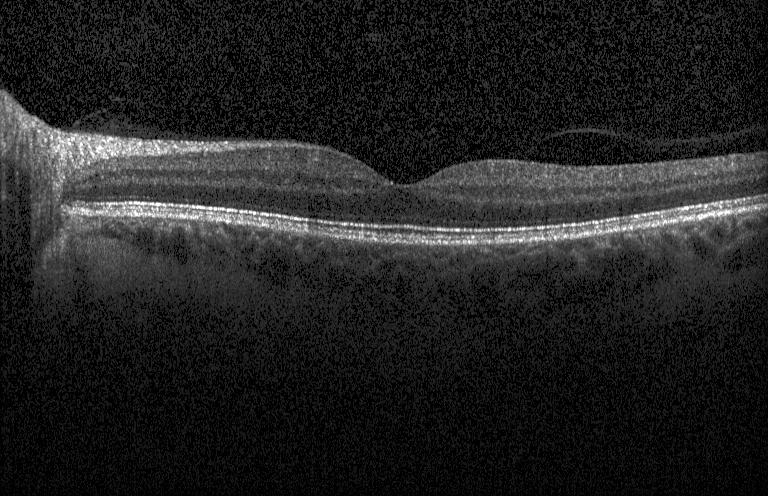
Macular OCT: no evidence of choroidal neovascularization, diabetic macular edema, or drusen.